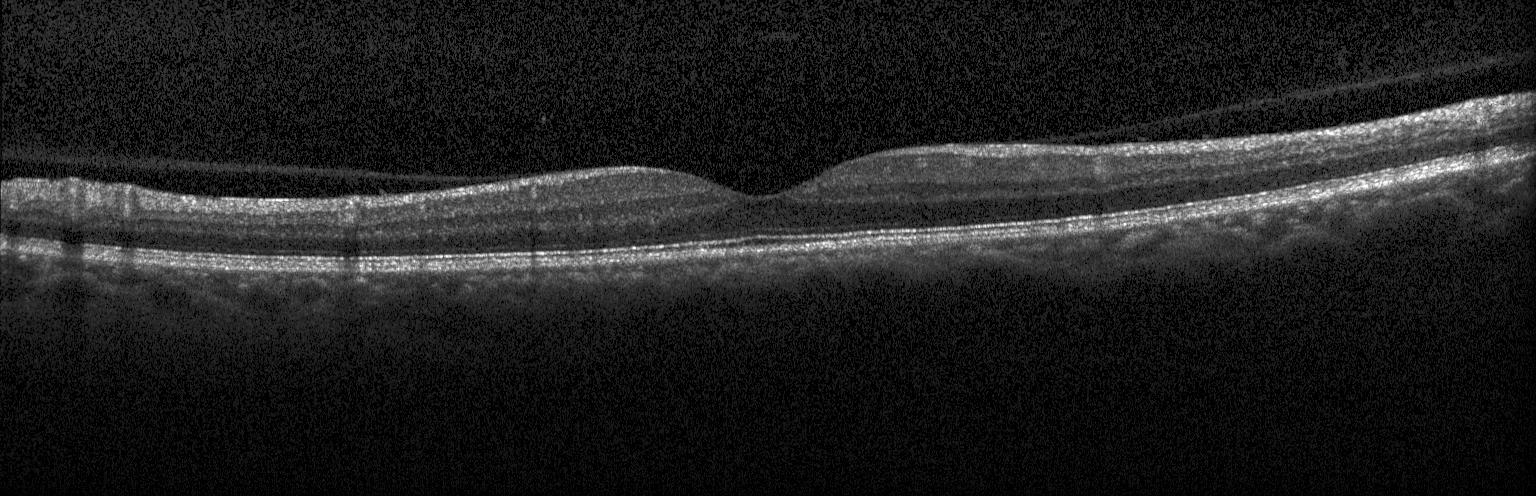

This B-scan demonstrates no choroidal neovascularization, no diabetic macular edema, and no drusen.